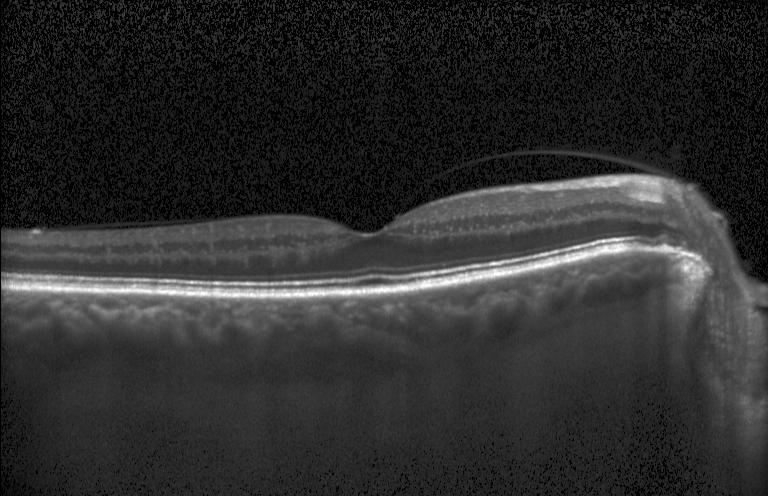

Retinal OCT cross-section.
Macular OCT: neither CNV, DME, nor drusen.